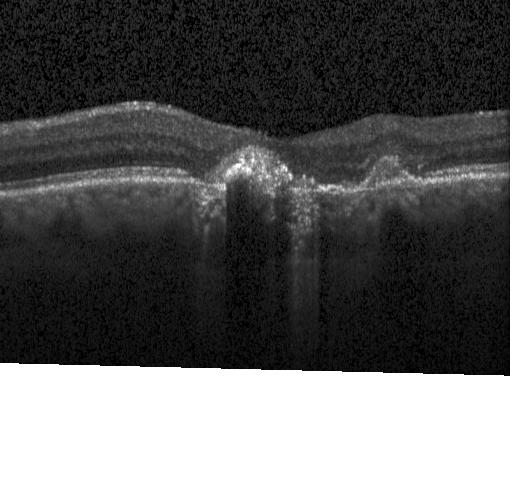
OCT scan showing CNV.